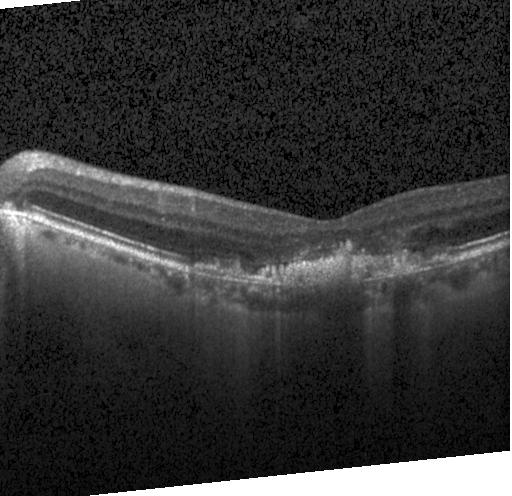
OCT line scan. Acquired on a Heidelberg Spectralis.
Diagnosis: a choroidal neovascular membrane.